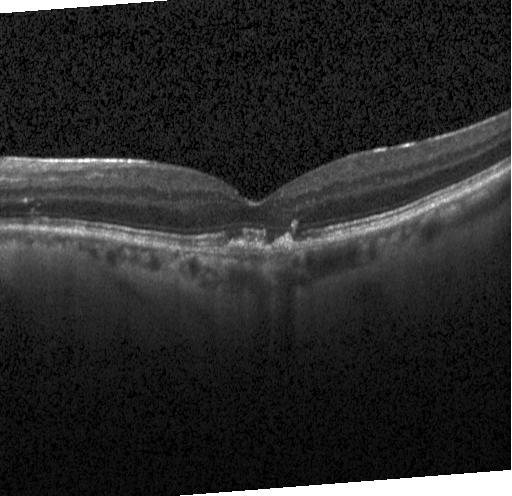

OCT B-scan. Diagnosis: choroidal neovascularization.